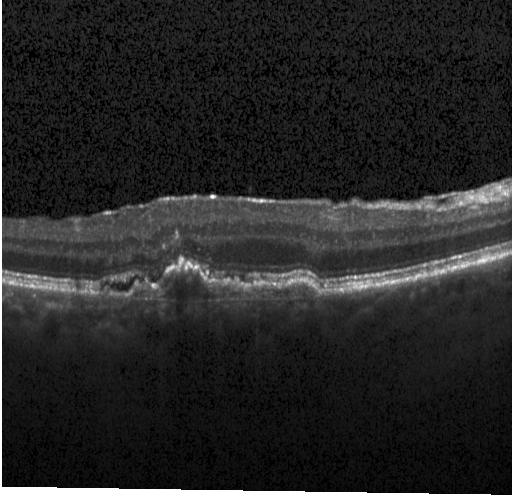 A choroidal neovascular membrane.